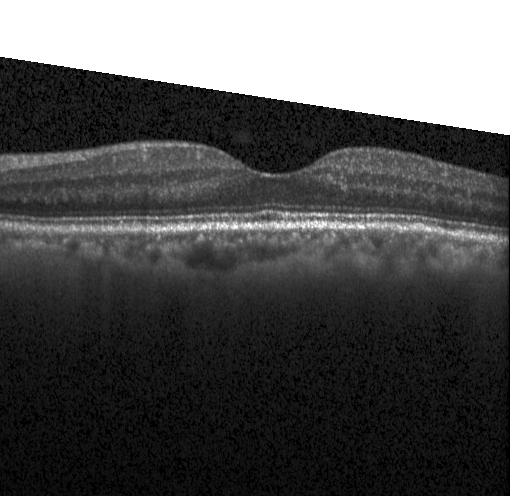 OCT line scan — The scan shows no evidence of CNV, DME, or drusen.